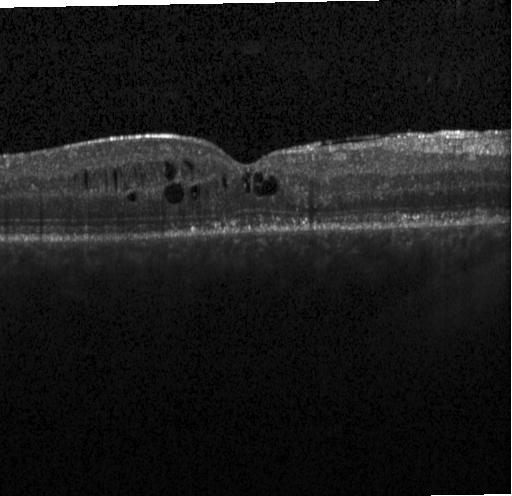
Dx: diabetic macular edema.